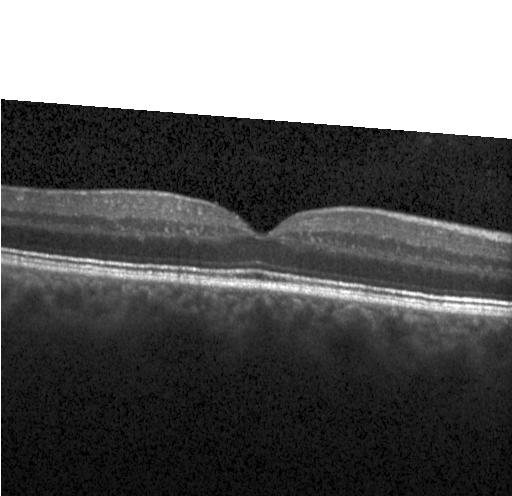

Optical coherence tomography scan — Diagnosis: no choroidal neovascularization, no diabetic macular edema, and no drusen.